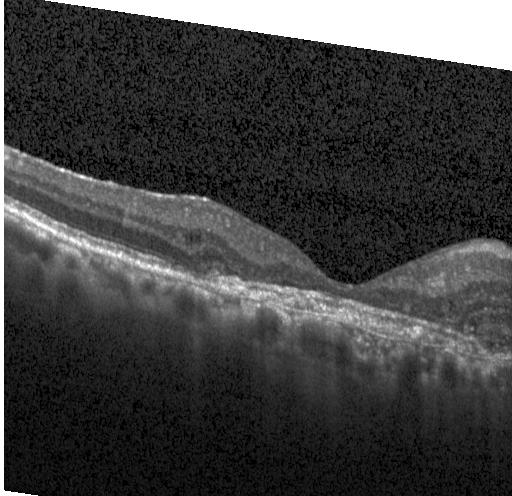 OCT line scan. Horizontal scan through the fovea — Assessment: a choroidal neovascular membrane.